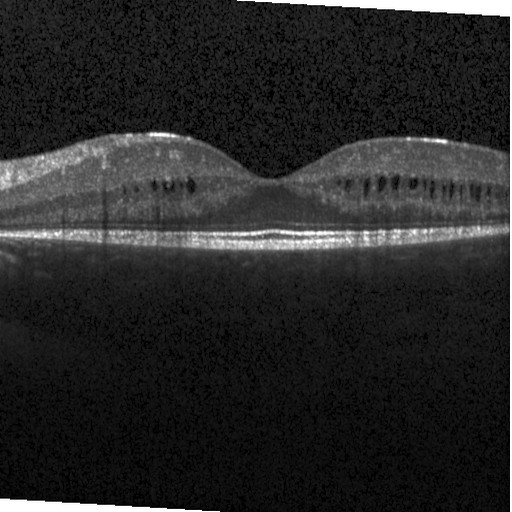

DME.